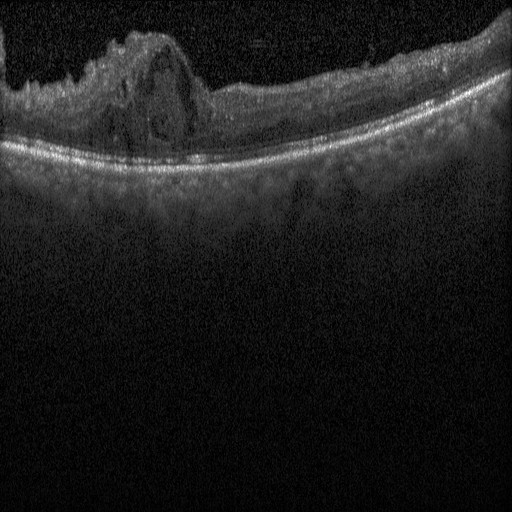
Dx: DME.